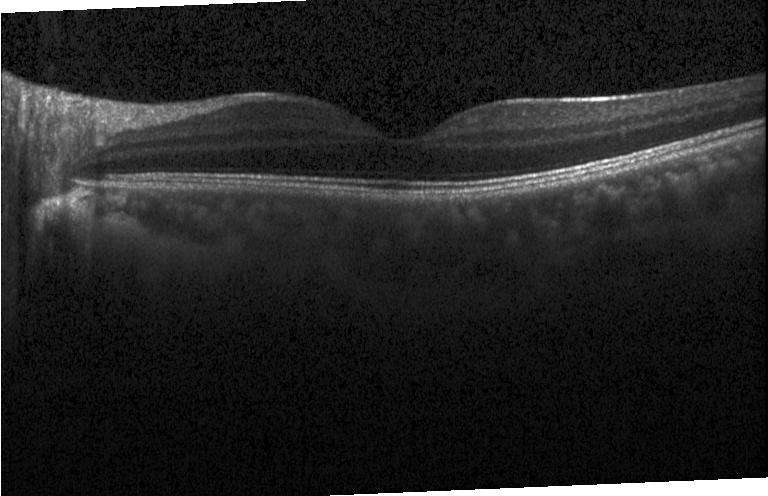

Horizontal scan through the fovea. Acquired on a Heidelberg Spectralis. Spectral-domain optical coherence tomography. OCT B-scan — Finding: neither choroidal neovascularization, diabetic macular edema, nor drusen.